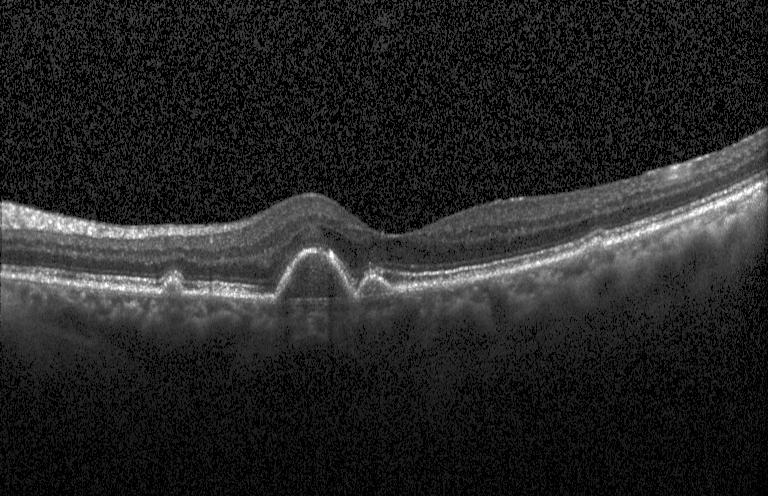

Retinal OCT B-scan — Impression: drusen.